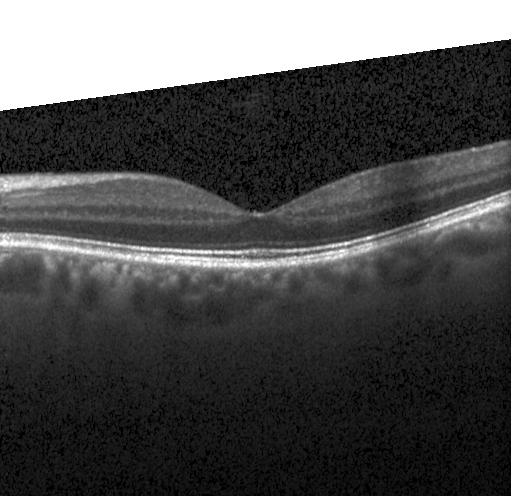
Retinal OCT cross-section.
Finding: neither choroidal neovascularization, diabetic macular edema, nor drusen.